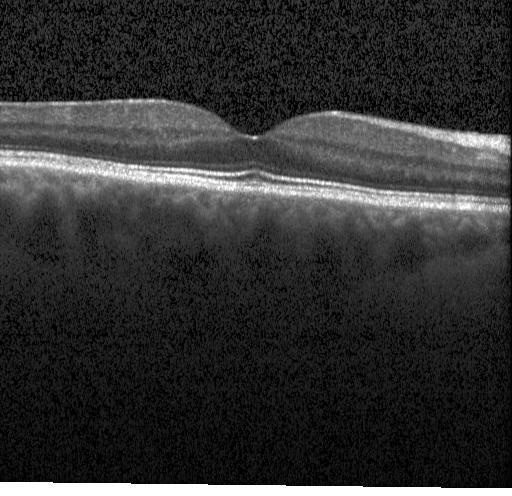
Centered on the fovea, retinal OCT B-scan, spectral-domain optical coherence tomography, Heidelberg Spectralis. Diagnosis: no evidence of CNV, DME, or drusen.